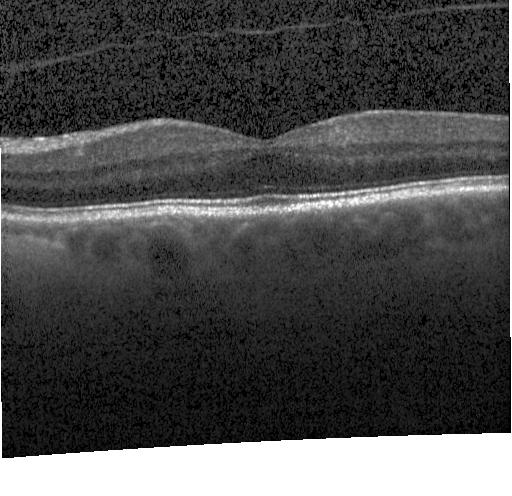

Optical coherence tomography scan · acquired on a Heidelberg Spectralis · SD-OCT. Dx: no CNV, DME, or drusen.